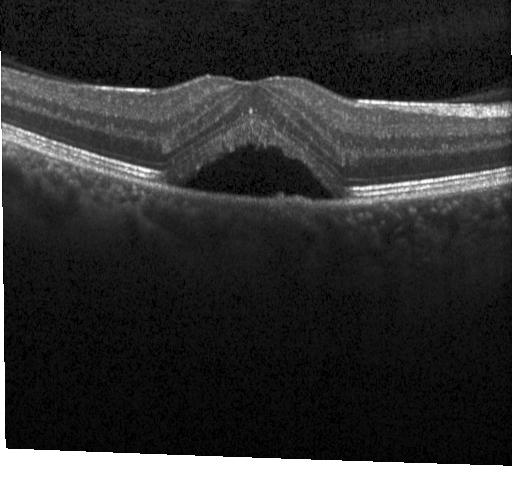 Impression: choroidal neovascularization.